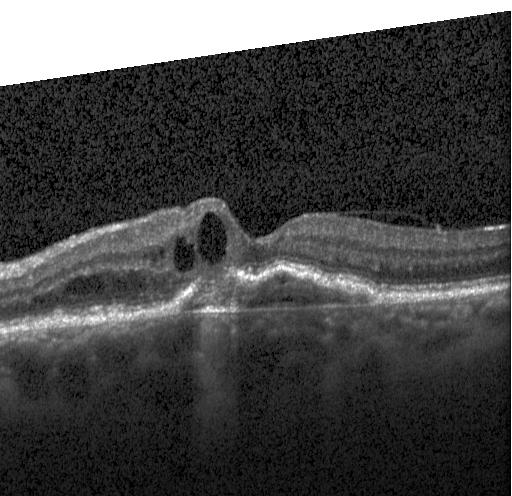
Optical coherence tomography B-scan
Finding: choroidal neovascularization (CNV).